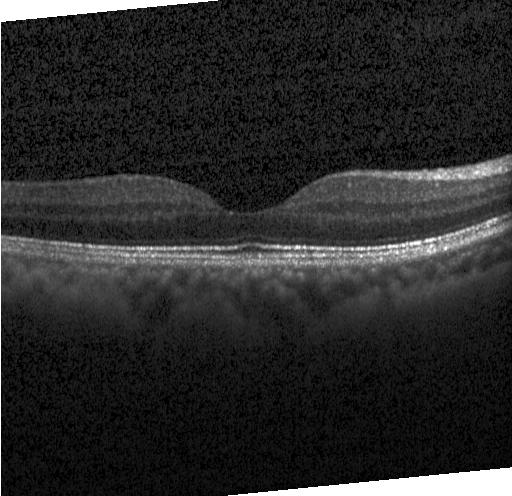
Dx: no evidence of choroidal neovascularization, diabetic macular edema, or drusen.